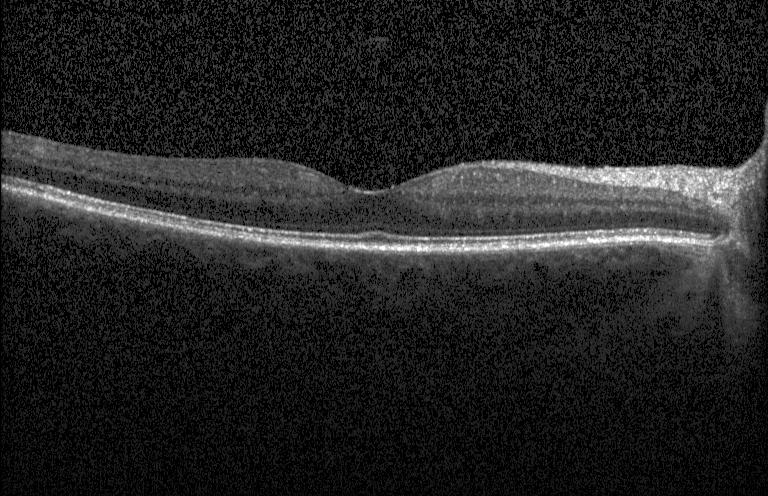 Spectral-domain OCT B-scan: no evidence of choroidal neovascularization, diabetic macular edema, or drusen.